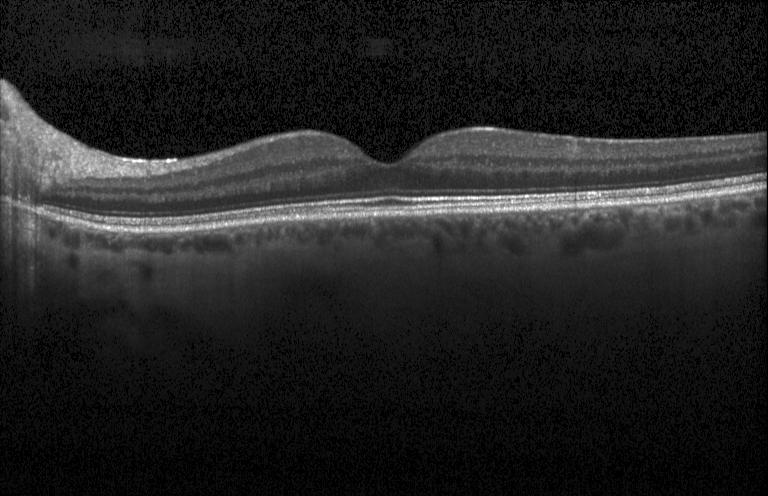
This B-scan demonstrates no CNV, no DME, and no drusen.